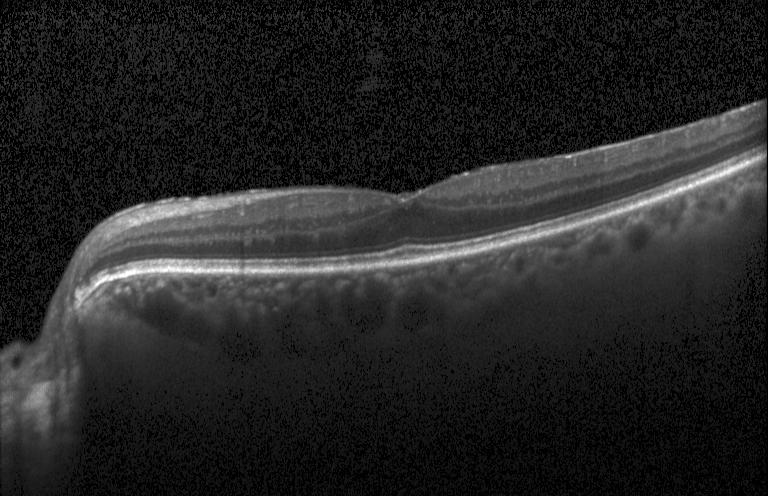
Spectral-domain OCT · horizontal scan through the fovea · OCT B-scan.
Diagnosis: no CNV, DME, or drusen.